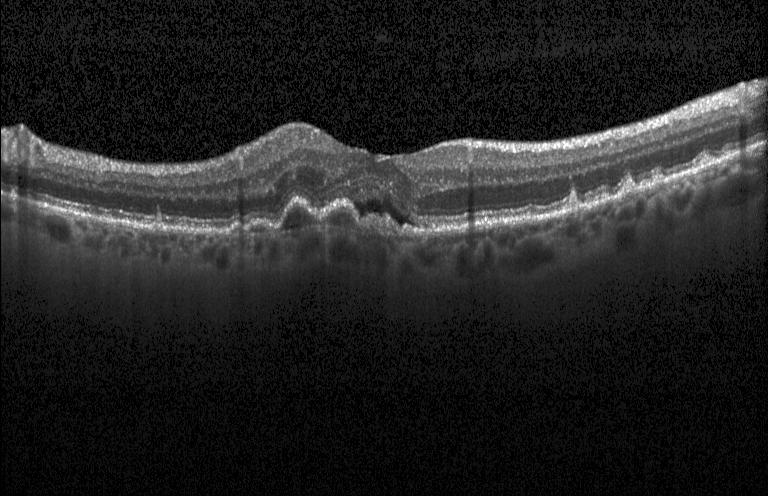 Instrument: Heidelberg Spectralis, optical coherence tomography scan, horizontal scan through the fovea, SD-OCT. Impression: a choroidal neovascular membrane.